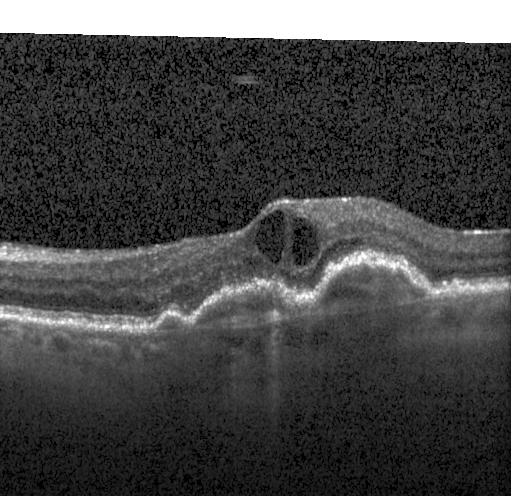
Optical coherence tomography B-scan. Diagnosis: a choroidal neovascular membrane.